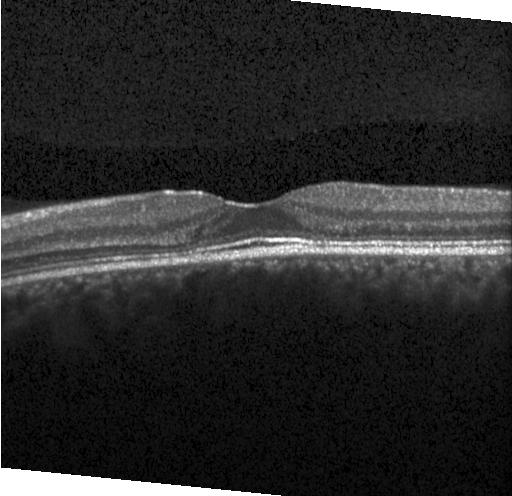 OCT B-scan. No evidence of choroidal neovascularization, diabetic macular edema, or drusen.